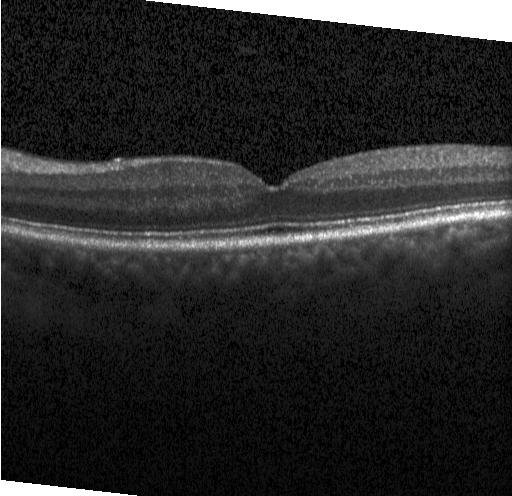
Heidelberg Spectralis, retinal OCT cross-section
Finding: no choroidal neovascularization, no diabetic macular edema, and no drusen.